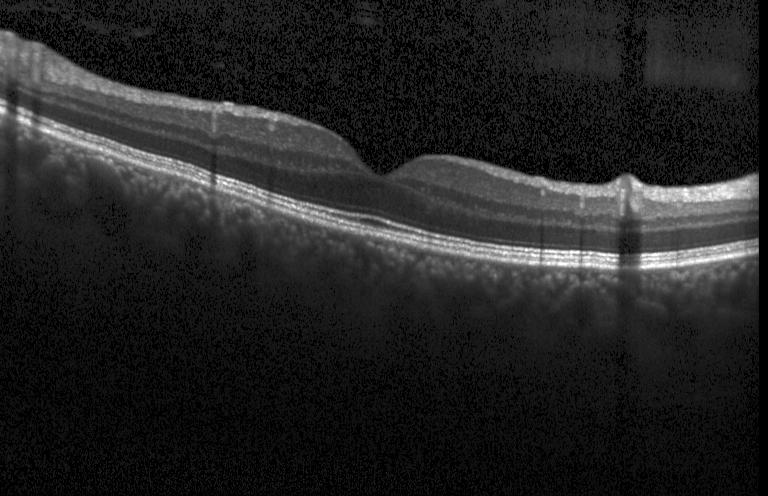 OCT finding: neither choroidal neovascularization, diabetic macular edema, nor drusen.